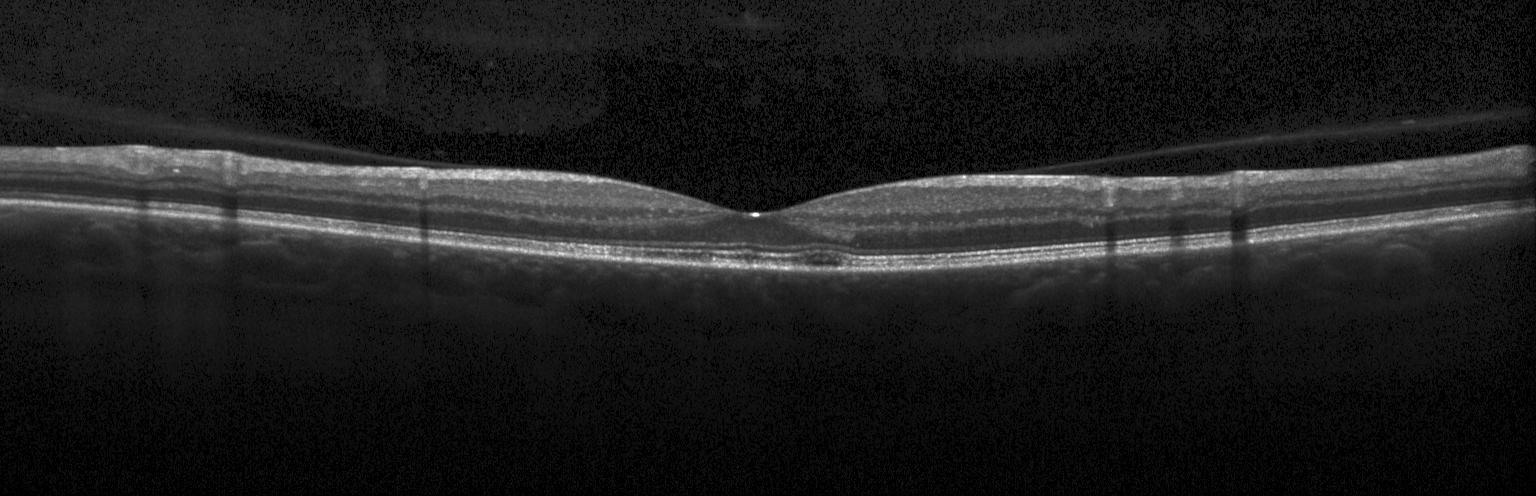
Optical coherence tomography B-scan. This B-scan demonstrates no choroidal neovascularization, no diabetic macular edema, and no drusen.